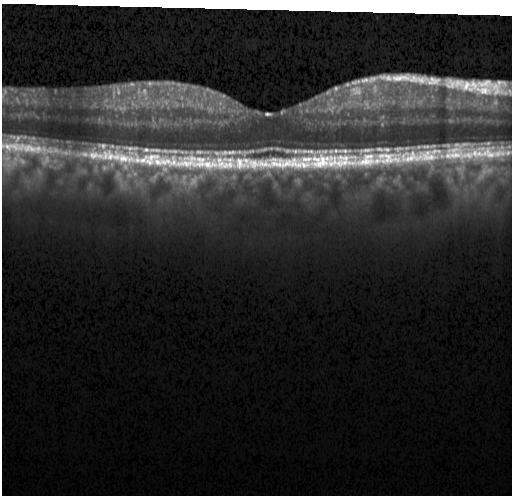
Spectral-domain OCT; OCT line scan; centered on the fovea; instrument: Heidelberg Spectralis
Macular OCT: no CNV, DME, or drusen.